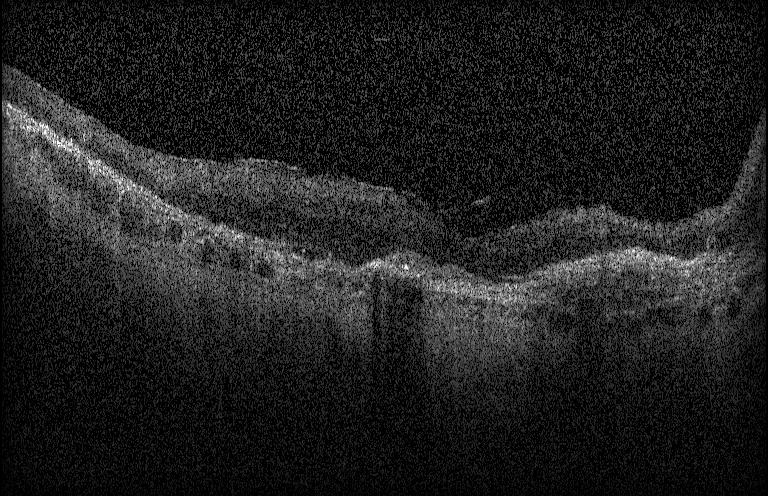 OCT finding: a choroidal neovascular membrane.